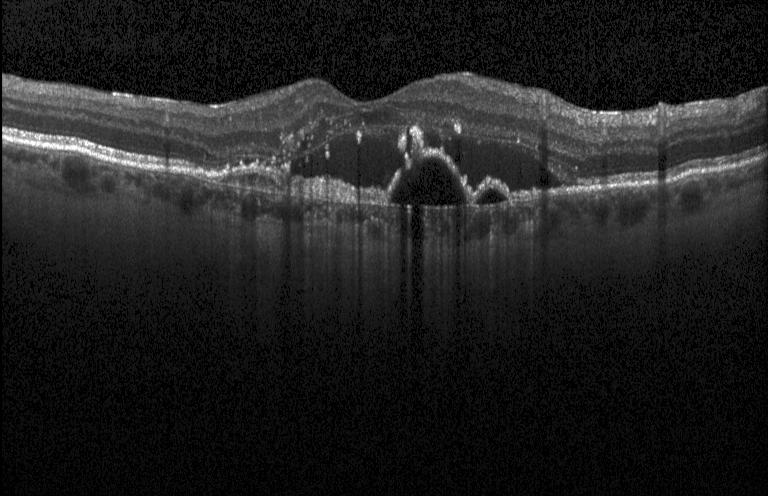
Retinal OCT B-scan · macular scan · Heidelberg Spectralis.
Finding: a choroidal neovascular membrane.